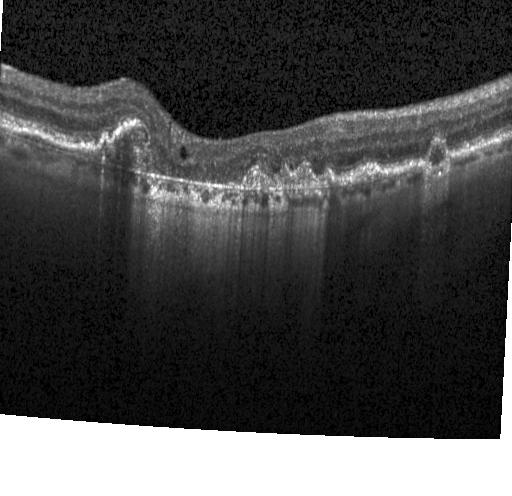 Optical coherence tomography scan; spectral-domain OCT; through the macula.
Diagnosis: a choroidal neovascular membrane.